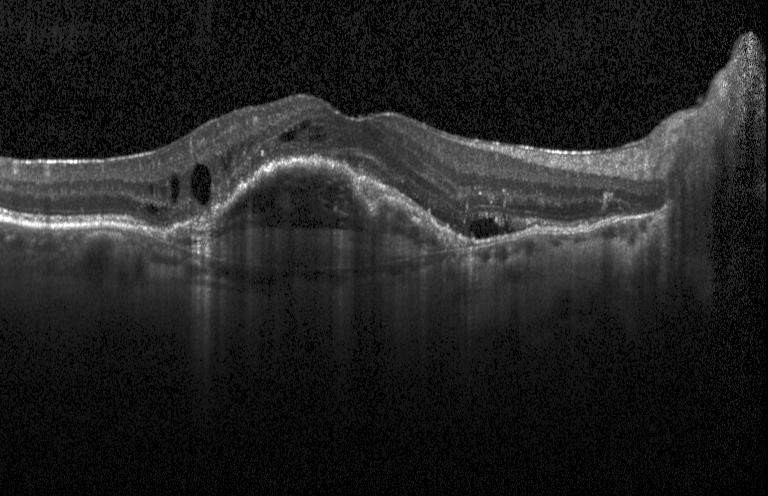
OCT B-scan. Diagnosis: a choroidal neovascular membrane.